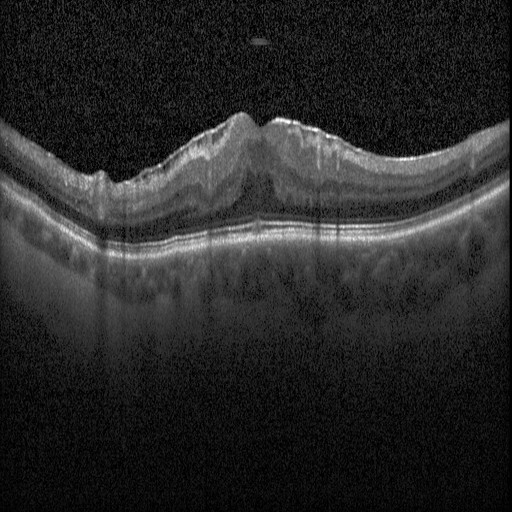 Optical coherence tomography B-scan — This B-scan demonstrates DME.